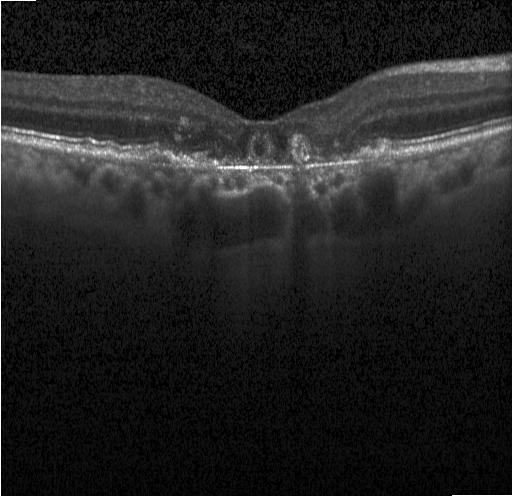 OCT B-scan. Impression: CNV.